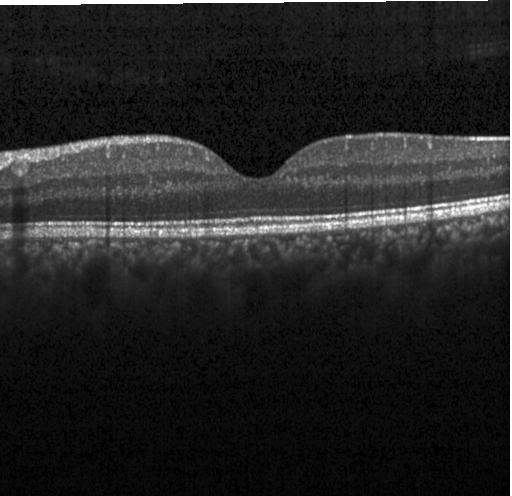
Optical coherence tomography B-scan; horizontal scan through the fovea; spectral-domain OCT; instrument: Heidelberg Spectralis — Finding: no choroidal neovascularization, no diabetic macular edema, and no drusen.